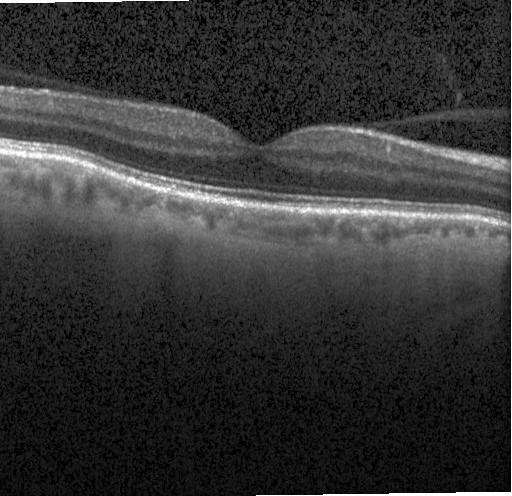

The scan shows no CNV, DME, or drusen.